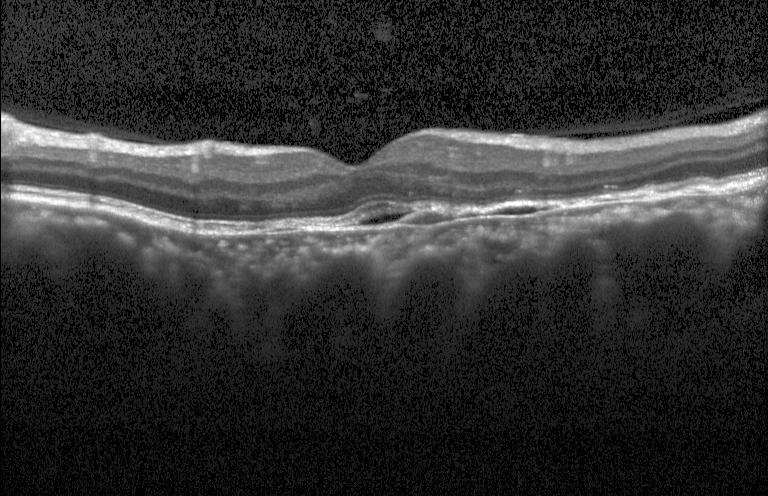
Impression: choroidal neovascularization.